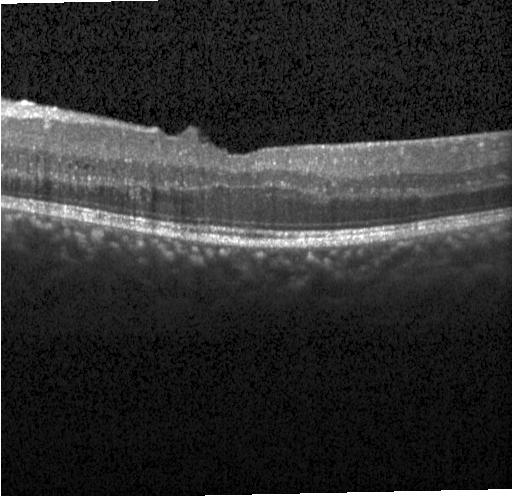 Macular OCT: diabetic macular edema.